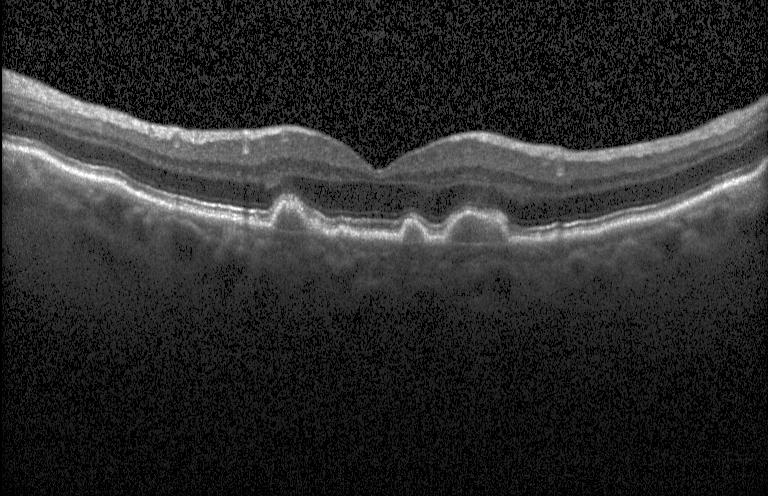
The scan shows multiple drusen.